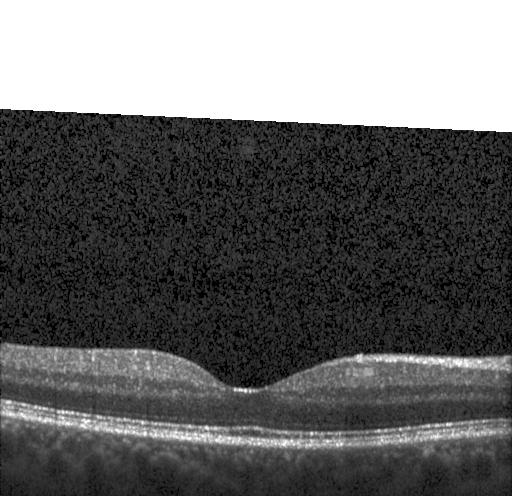

Fovea-centered · instrument: Heidelberg Spectralis · OCT B-scan · SD-OCT — No choroidal neovascularization, diabetic macular edema, or drusen.